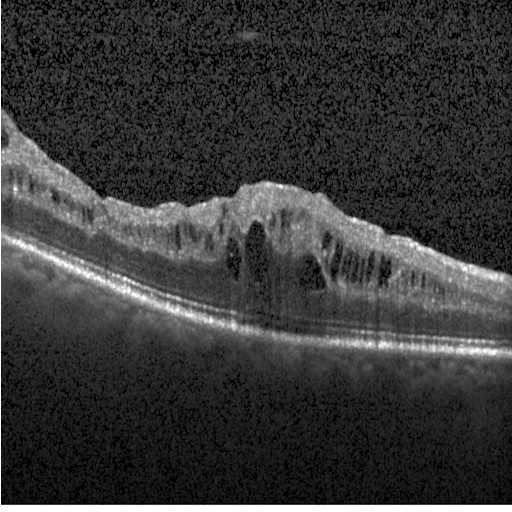 Optical coherence tomography B-scan, through the macula, spectral-domain optical coherence tomography, Heidelberg Spectralis OCT system. Finding: diabetic macular edema (DME).